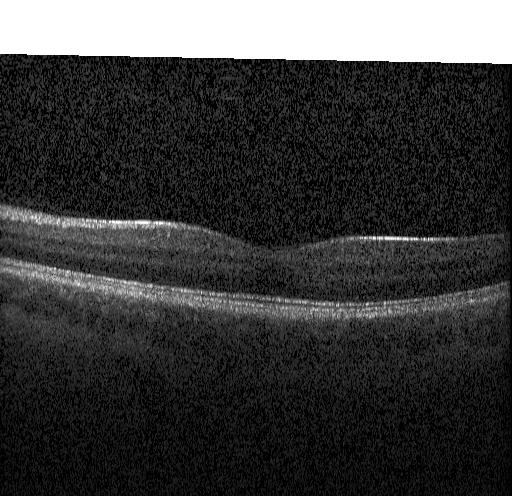

Spectral-domain OCT; OCT line scan — Finding: no choroidal neovascularization, no diabetic macular edema, and no drusen.